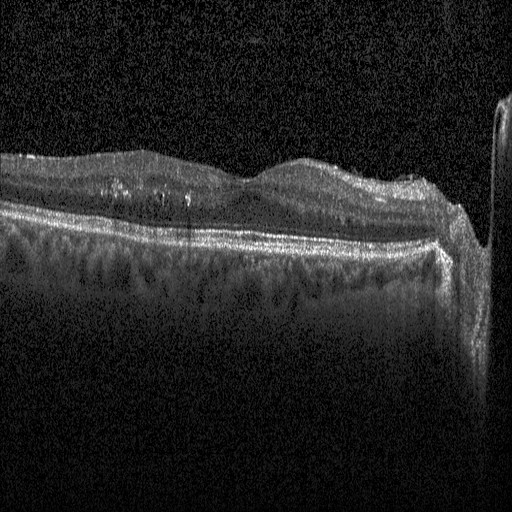 Finding: diabetic macular edema (DME).